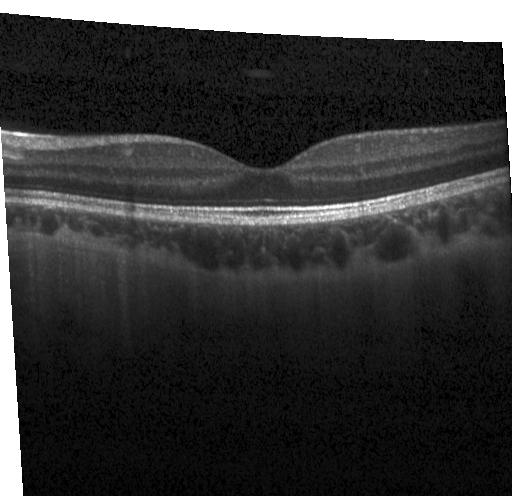

Impression: neither choroidal neovascularization, diabetic macular edema, nor drusen.